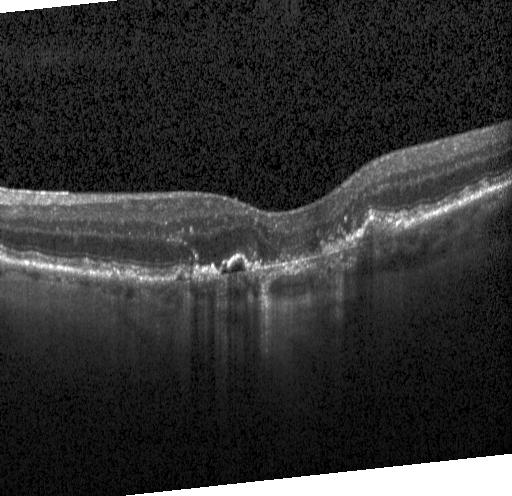 Optical coherence tomography scan · instrument: Heidelberg Spectralis · spectral-domain OCT · through the macula. Dx: a choroidal neovascular membrane.